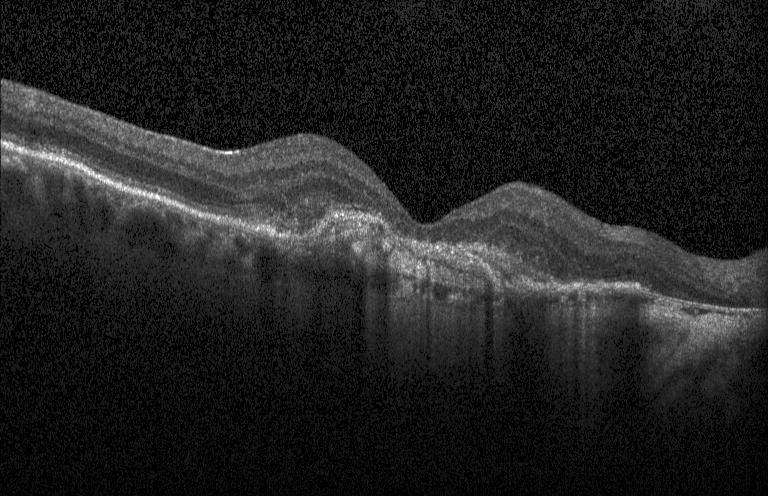 Fovea-centered · spectral-domain OCT · OCT line scan · Heidelberg Spectralis OCT system
Dx: choroidal neovascularization.